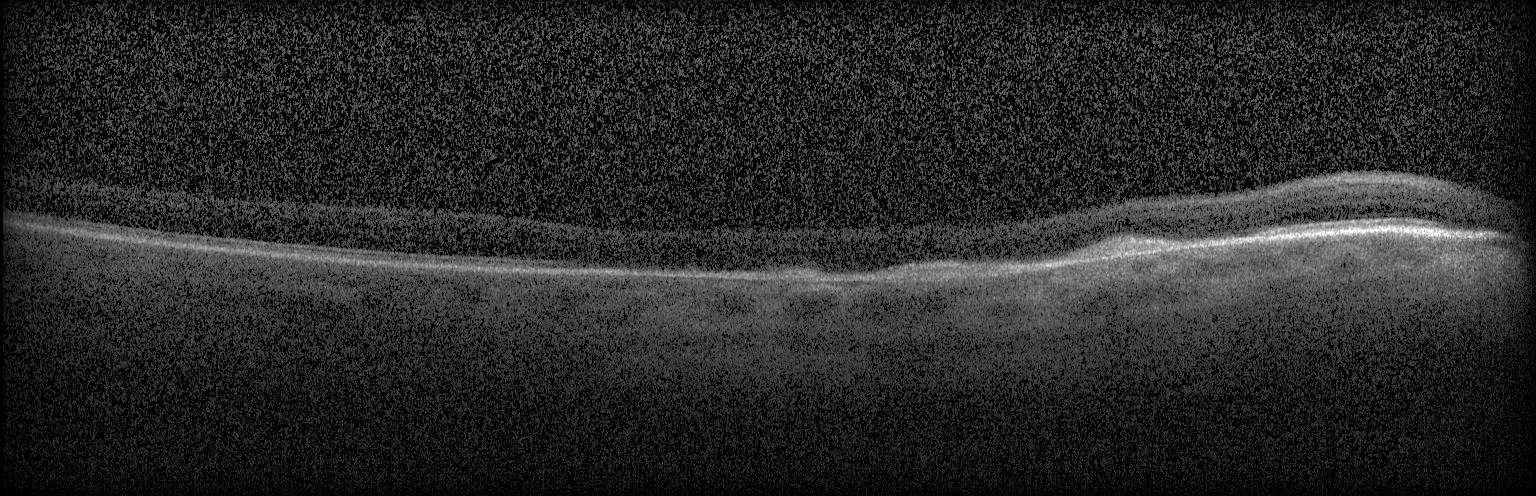 OCT line scan
Impression: a choroidal neovascular membrane.